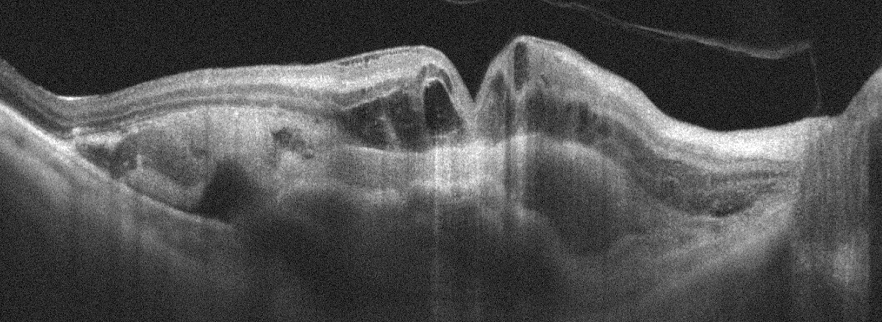 Acquired on an Optovue Avanti RTVue XR · optical coherence tomography B-scan — Dx: AMD.